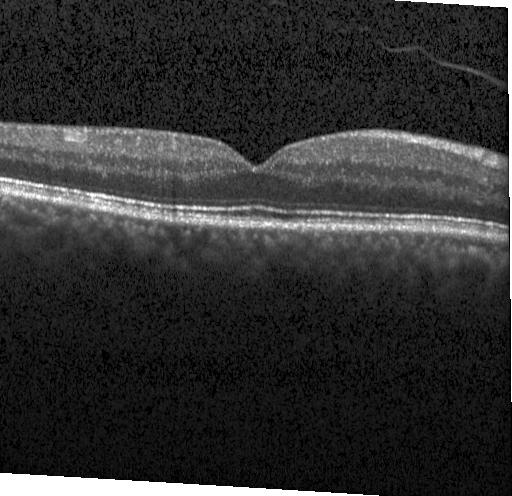

Retinal OCT cross-section
Impression: no CNV, DME, or drusen.